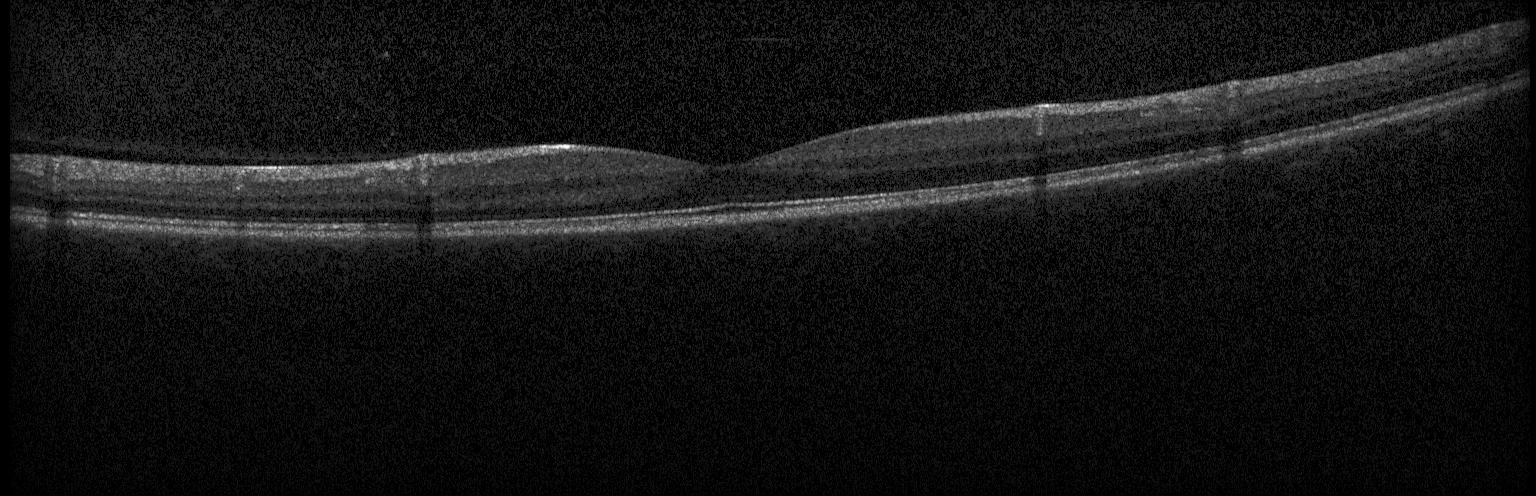
Acquired on a Heidelberg Spectralis, retinal OCT B-scan
This B-scan demonstrates no choroidal neovascularization, diabetic macular edema, or drusen.